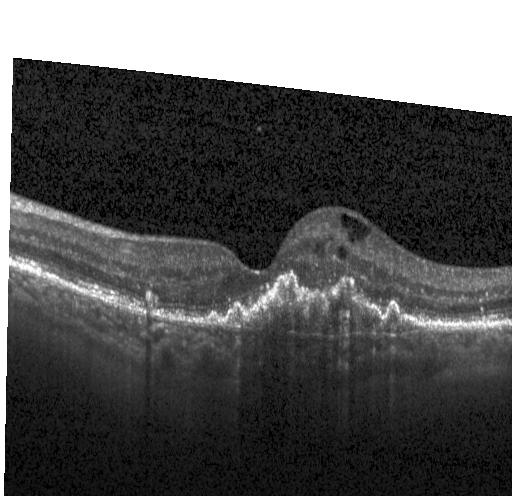
Optical coherence tomography scan; through the macula; Heidelberg Spectralis.
Impression: CNV.